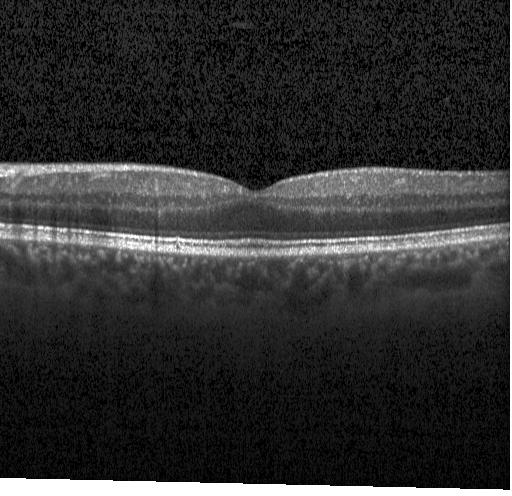

Optical coherence tomography scan · spectral-domain OCT. Finding: no CNV, no DME, and no drusen.